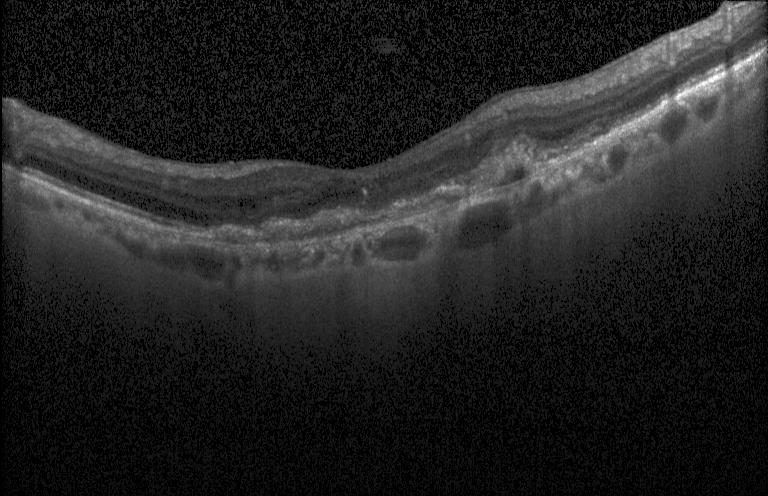

Spectral-domain optical coherence tomography · retinal OCT cross-section
Finding: choroidal neovascularization.